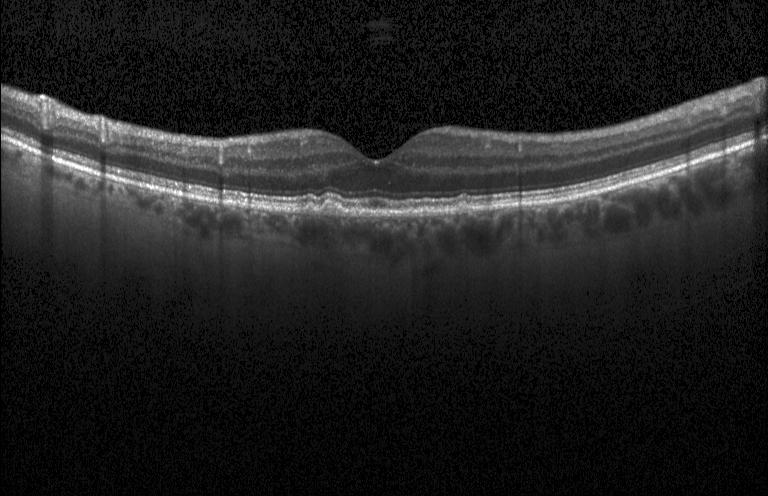
Diagnosis: drusen.